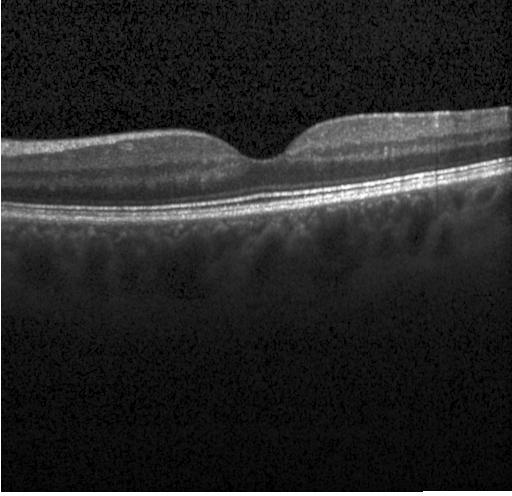

OCT B-scan
Assessment: no choroidal neovascularization, no diabetic macular edema, and no drusen.